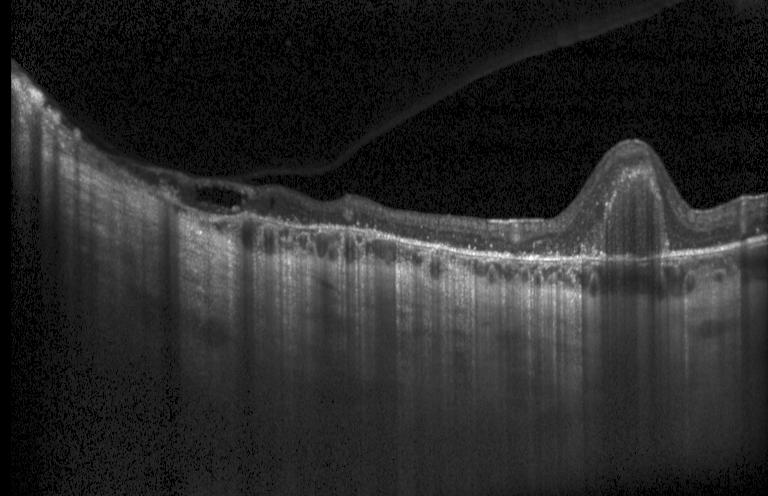

Centered on the fovea. Retinal OCT B-scan — This B-scan demonstrates choroidal neovascularization.